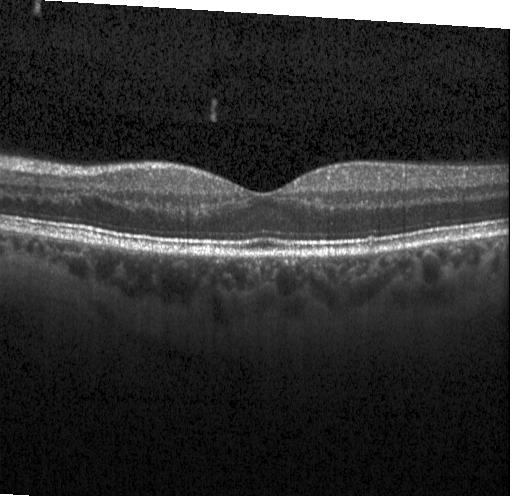

Centered on the fovea; optical coherence tomography scan; spectral-domain OCT; Heidelberg Spectralis OCT system.
The scan shows no evidence of CNV, DME, or drusen.